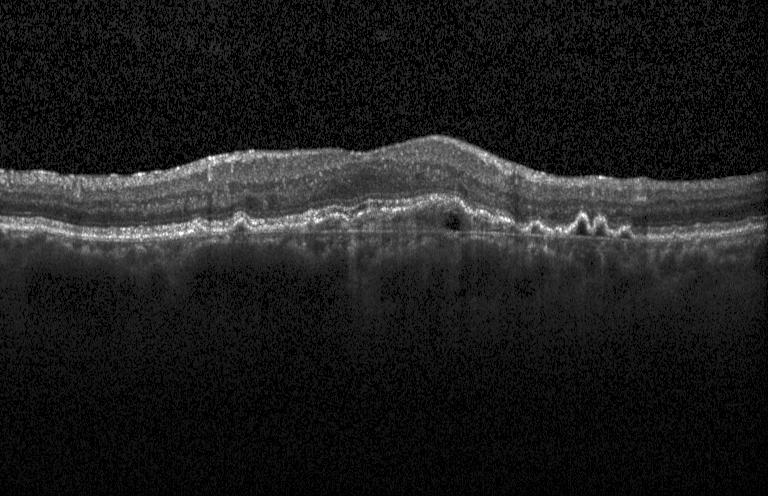

Optical coherence tomography B-scan — Diagnosis: choroidal neovascularization (CNV).